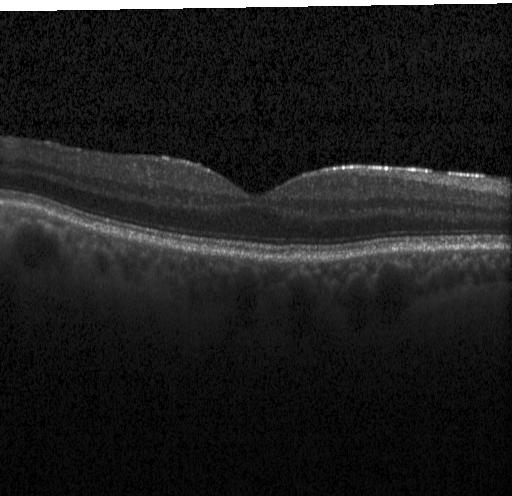 Optical coherence tomography B-scan. Spectral-domain OCT.
No CNV, no DME, and no drusen.